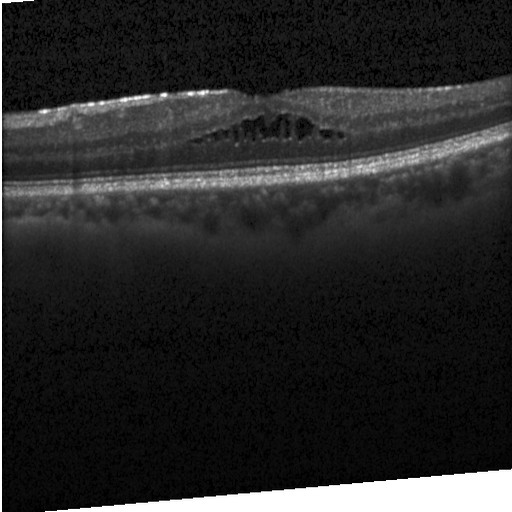
Dx: diabetic macular edema.